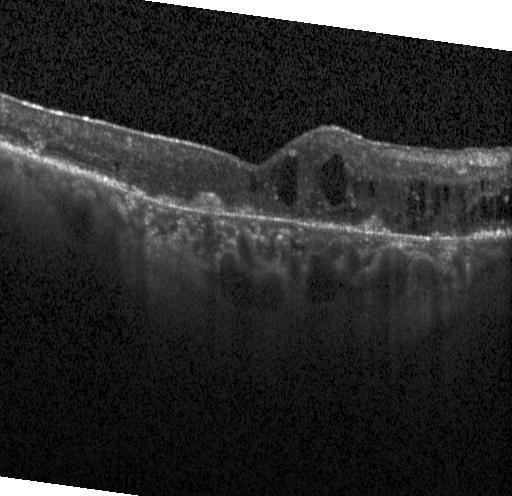

Spectral-domain OCT · OCT line scan · through the macula · Heidelberg Spectralis. The scan shows a choroidal neovascular membrane.